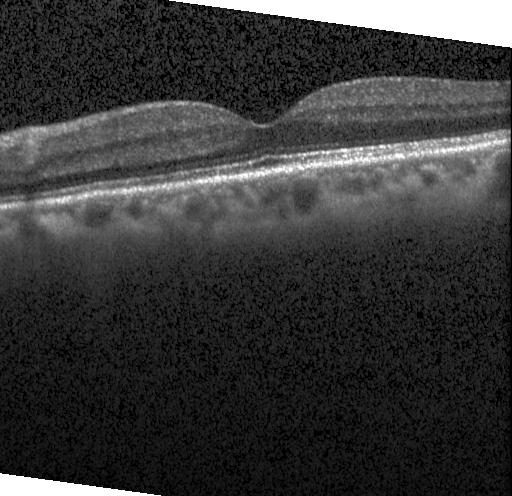

OCT line scan
No CNV, DME, or drusen.